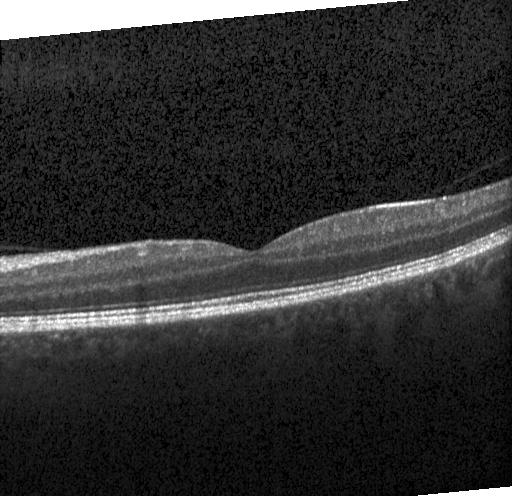
Spectral-domain OCT. Centered on the fovea. Retinal OCT cross-section.
Finding: neither choroidal neovascularization, diabetic macular edema, nor drusen.